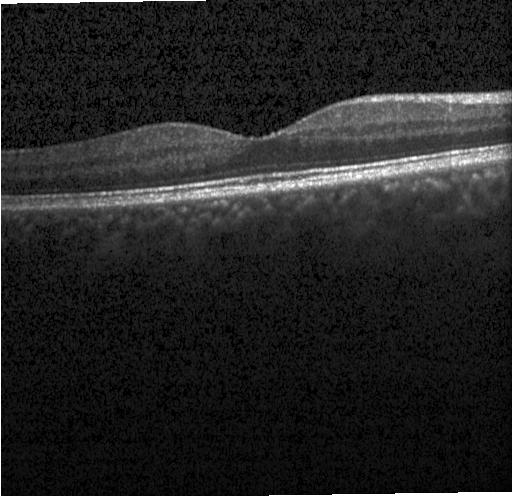
OCT B-scan
Diagnosis: neither CNV, DME, nor drusen.